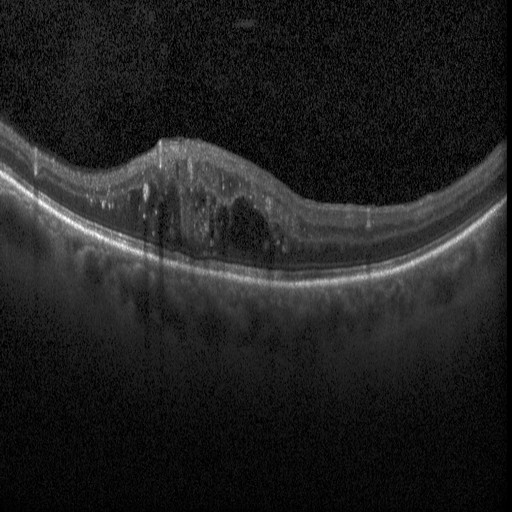

Diagnosis: diabetic macular edema.